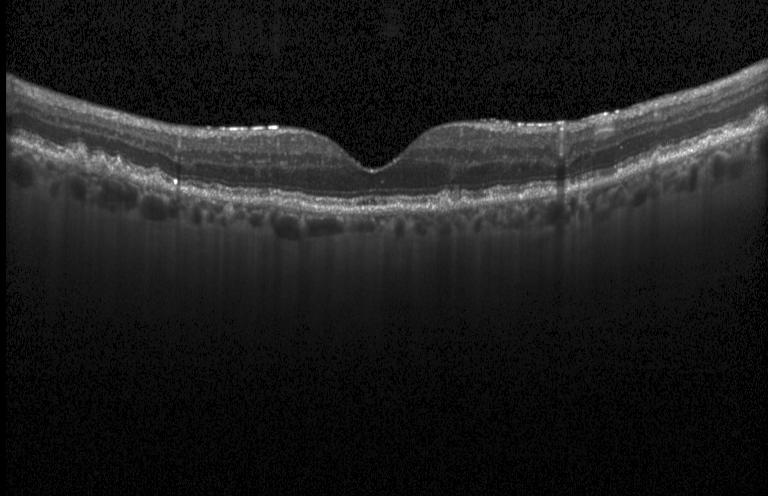
Horizontal scan through the fovea; acquired on a Heidelberg Spectralis; SD-OCT; retinal OCT B-scan.
Finding: multiple drusen.